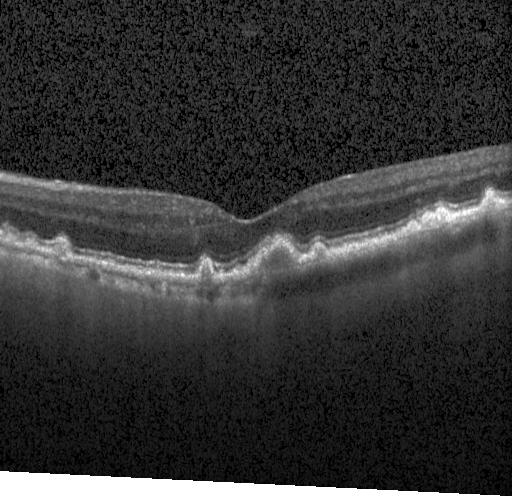

Acquired on a Heidelberg Spectralis, optical coherence tomography scan, centered on the fovea. This B-scan demonstrates multiple drusen.